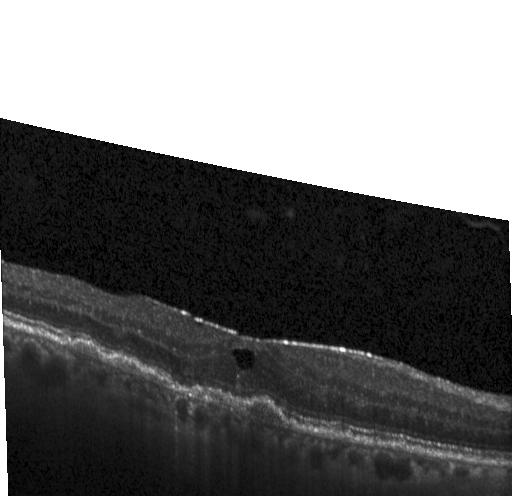 Optical coherence tomography B-scan; through the macula. OCT finding: a choroidal neovascular membrane.